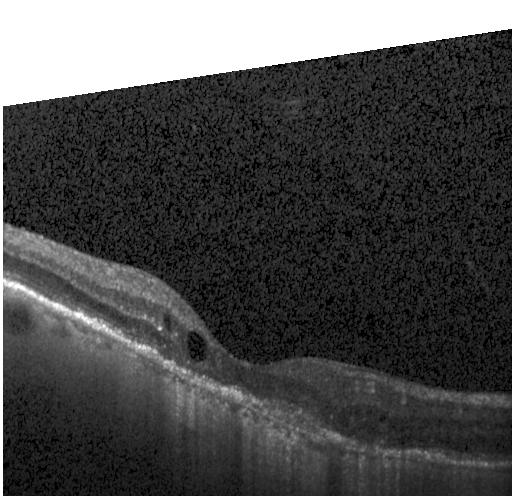

Heidelberg Spectralis OCT system; macular scan; optical coherence tomography scan; spectral-domain optical coherence tomography. The scan shows a choroidal neovascular membrane.